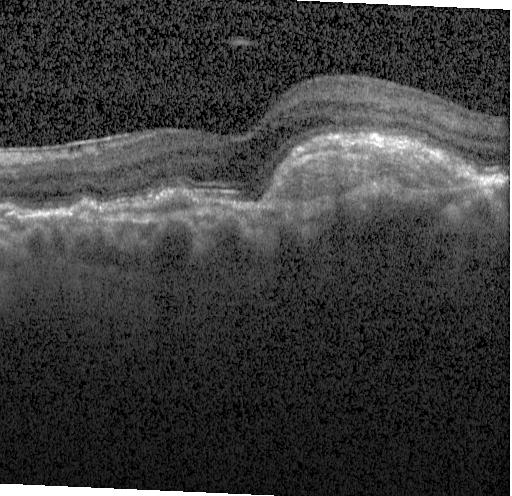

OCT line scan.
Dx: a choroidal neovascular membrane.